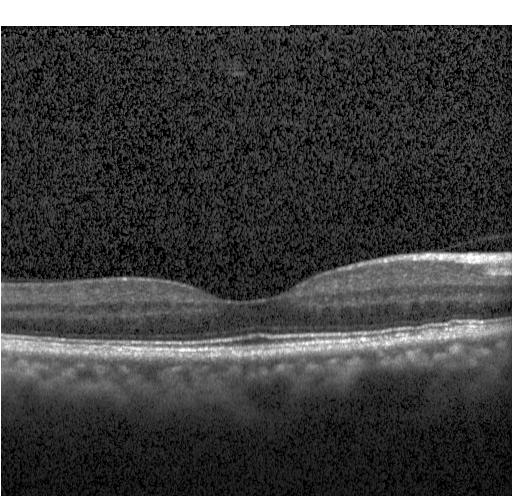
Spectral-domain OCT, OCT B-scan, macular scan — Finding: no choroidal neovascularization, no diabetic macular edema, and no drusen.